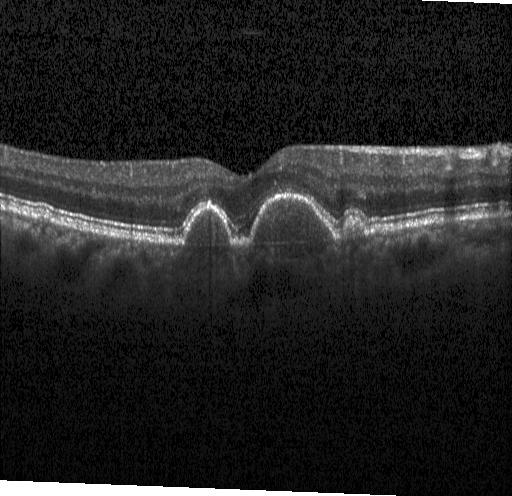 Impression: multiple drusen.